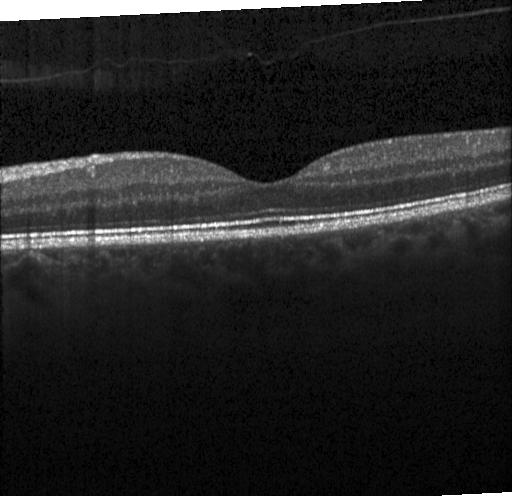
Finding: no choroidal neovascularization, no diabetic macular edema, and no drusen.